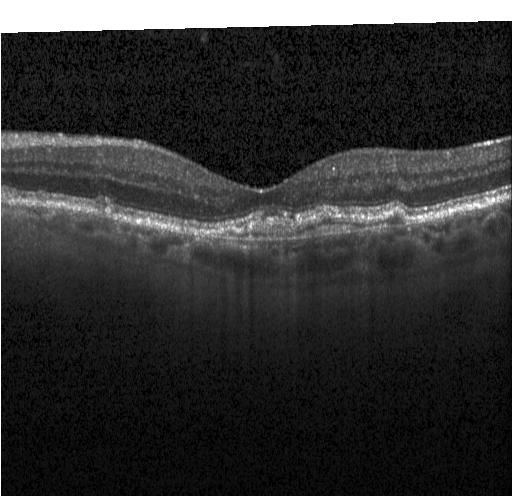
Spectral-domain OCT B-scan: a choroidal neovascular membrane.